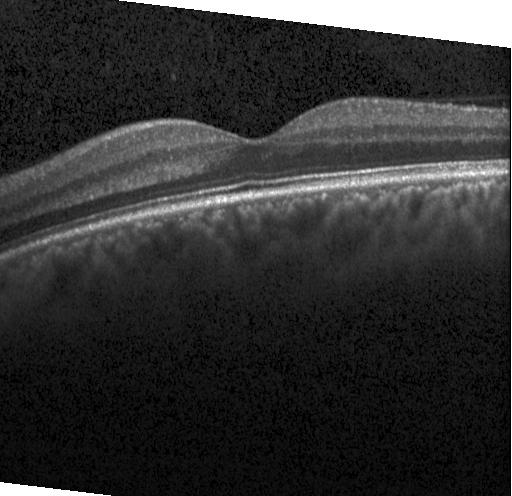
OCT B-scan showing no choroidal neovascularization, no diabetic macular edema, and no drusen.